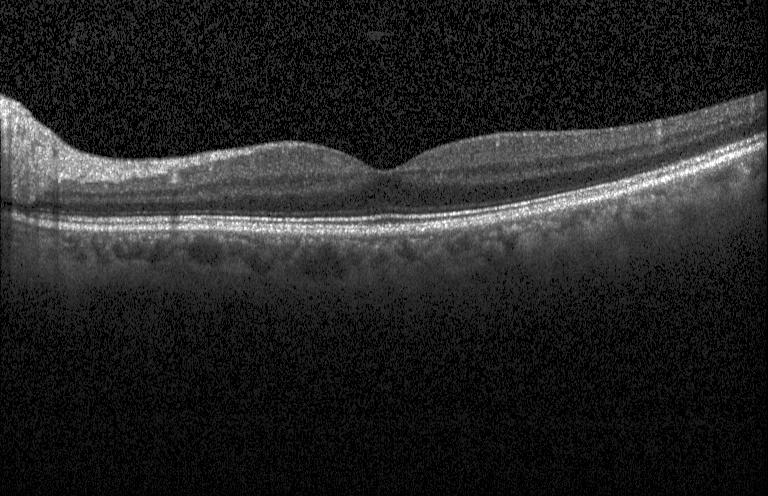

Spectral-domain optical coherence tomography · OCT line scan · macular scan
Finding: no evidence of choroidal neovascularization, diabetic macular edema, or drusen.